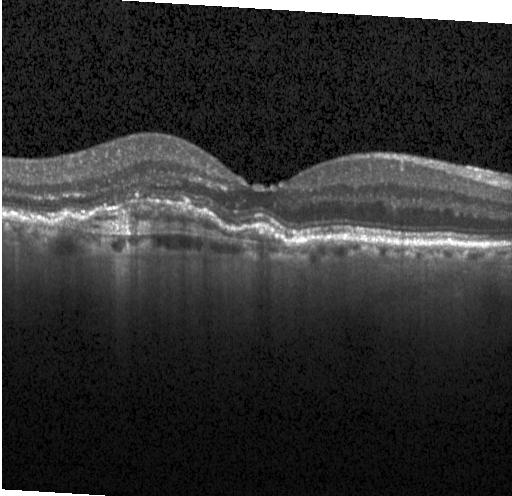 Optical coherence tomography B-scan.
The scan shows CNV.